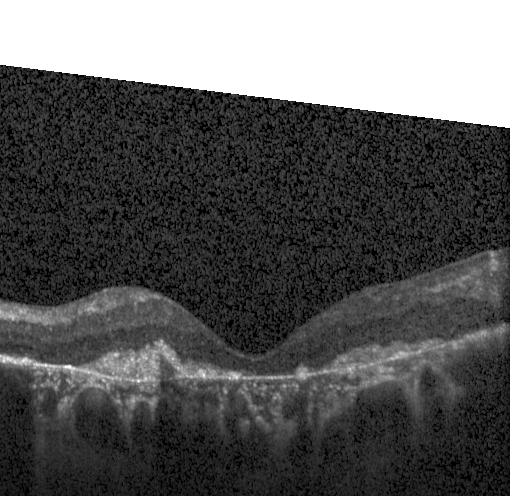

Optical coherence tomography scan; spectral-domain optical coherence tomography. Impression: choroidal neovascularization.